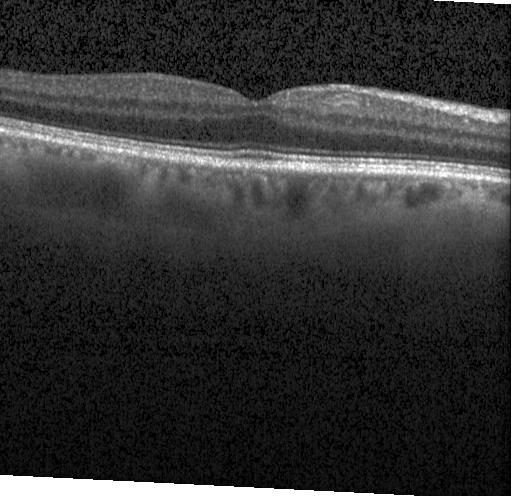

OCT B-scan, fovea-centered, Heidelberg Spectralis. Finding: no choroidal neovascularization, diabetic macular edema, or drusen.